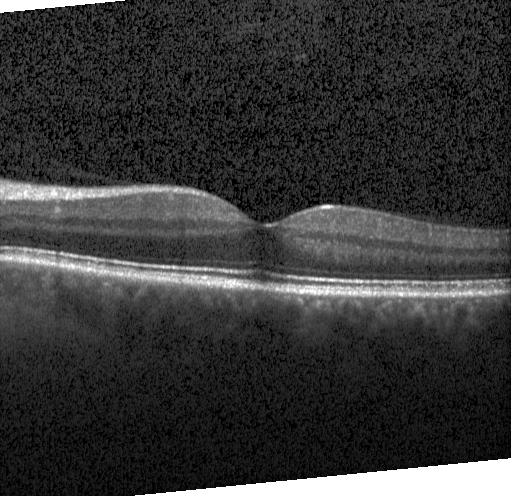
Macular OCT demonstrating no CNV, DME, or drusen.